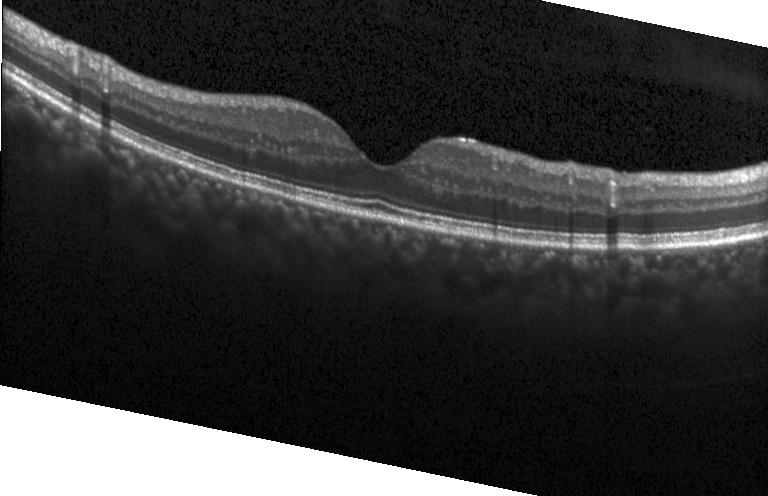
Acquired on a Heidelberg Spectralis, optical coherence tomography B-scan, centered on the fovea — Assessment: no choroidal neovascularization, diabetic macular edema, or drusen.